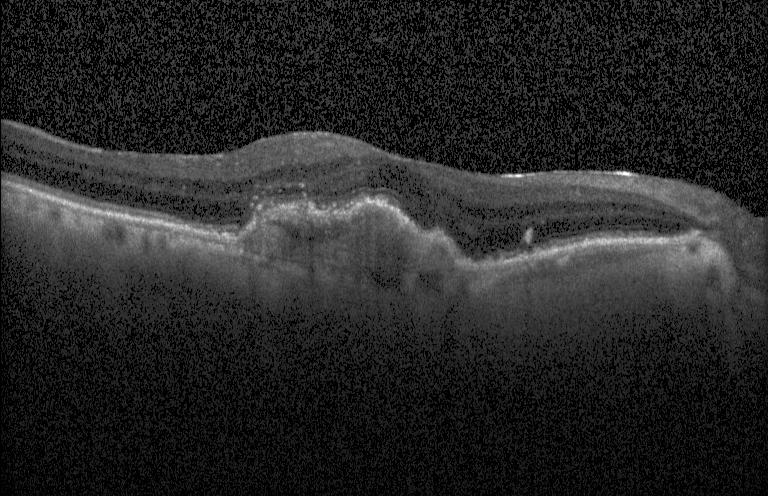

Retinal OCT cross-section.
Impression: choroidal neovascularization.